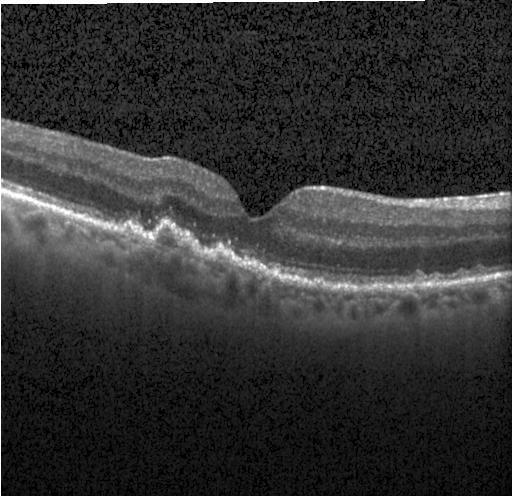 SD-OCT · retinal OCT cross-section · through the macula — Dx: sub-RPE drusenoid deposits.